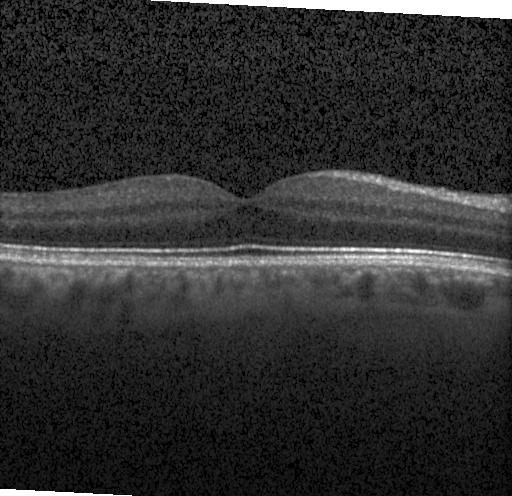 No choroidal neovascularization, no diabetic macular edema, and no drusen.